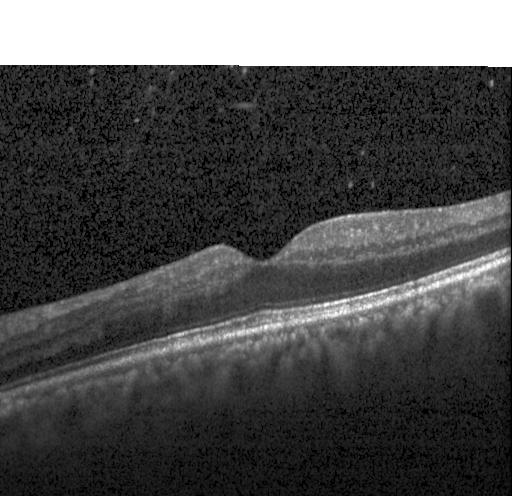 OCT B-scan, spectral-domain optical coherence tomography, centered on the fovea — This B-scan demonstrates no choroidal neovascularization, no diabetic macular edema, and no drusen.